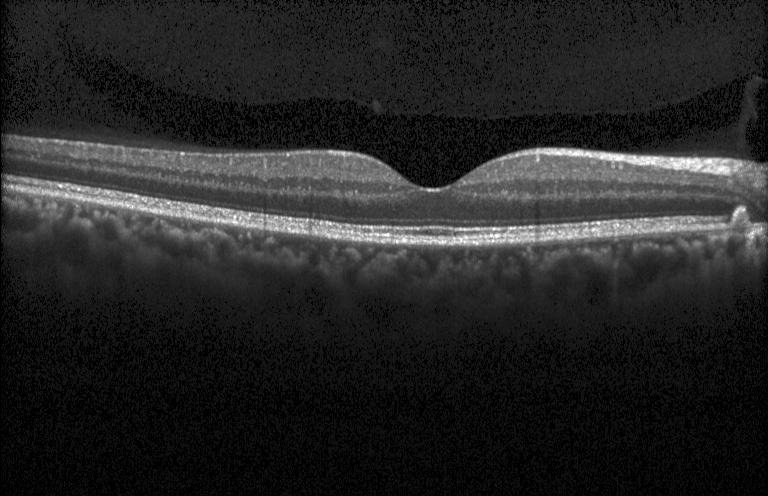

Optical coherence tomography scan.
Assessment: no evidence of choroidal neovascularization, diabetic macular edema, or drusen.